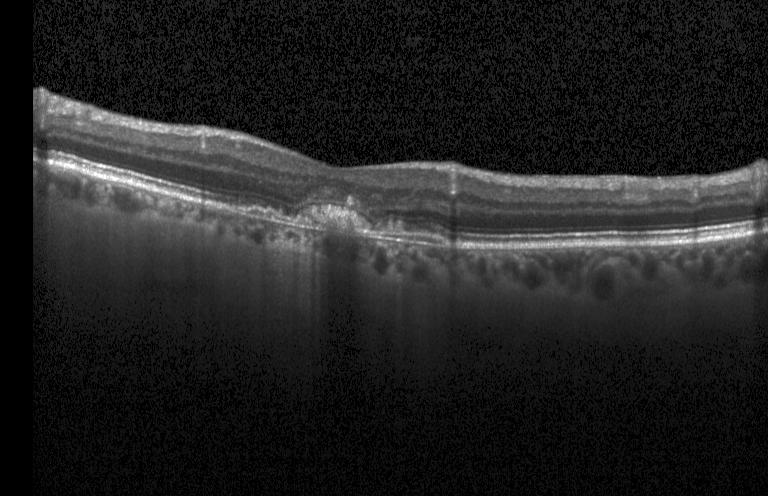
A choroidal neovascular membrane.